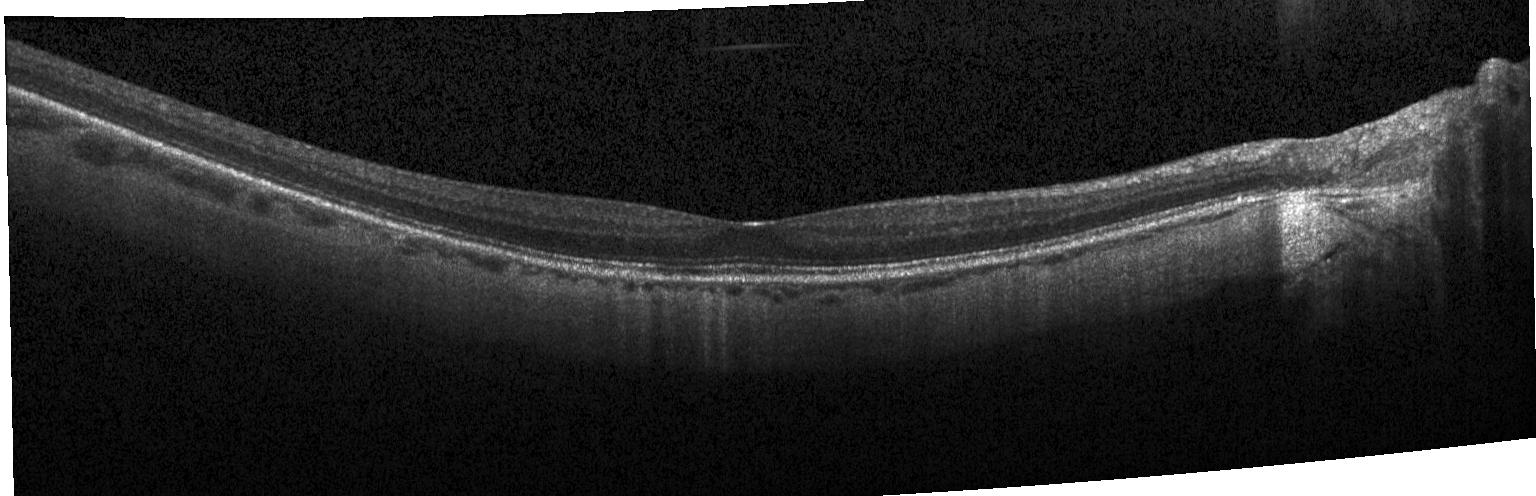 Acquired on a Heidelberg Spectralis · OCT B-scan · through the macula — Dx: neither CNV, DME, nor drusen.